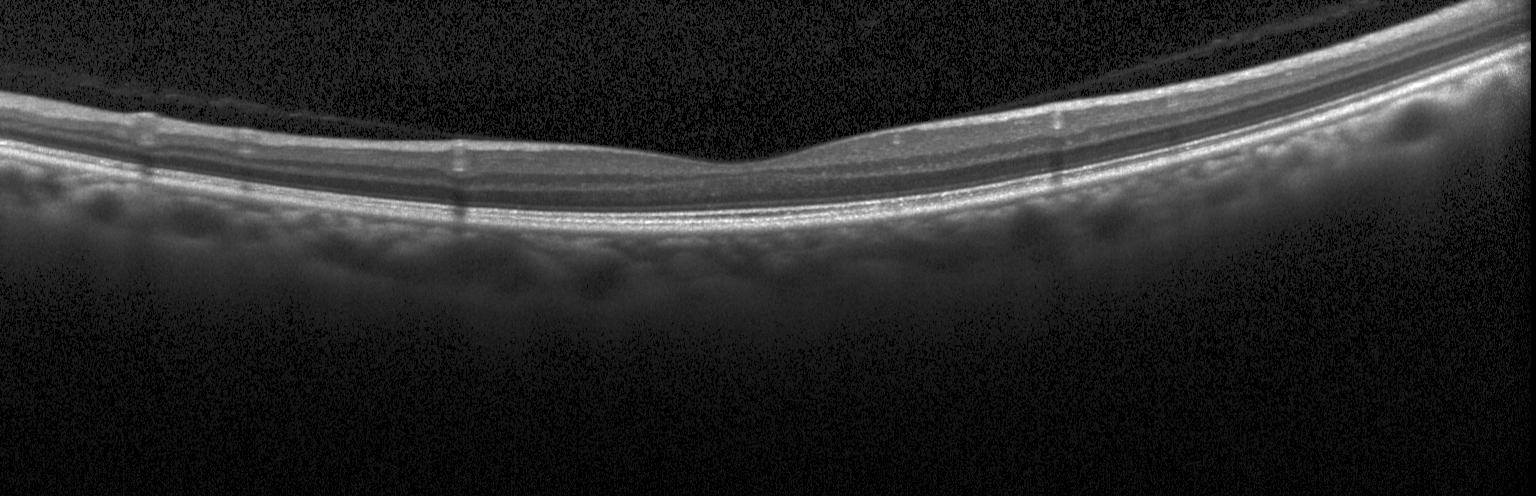
OCT scan showing no CNV, DME, or drusen.